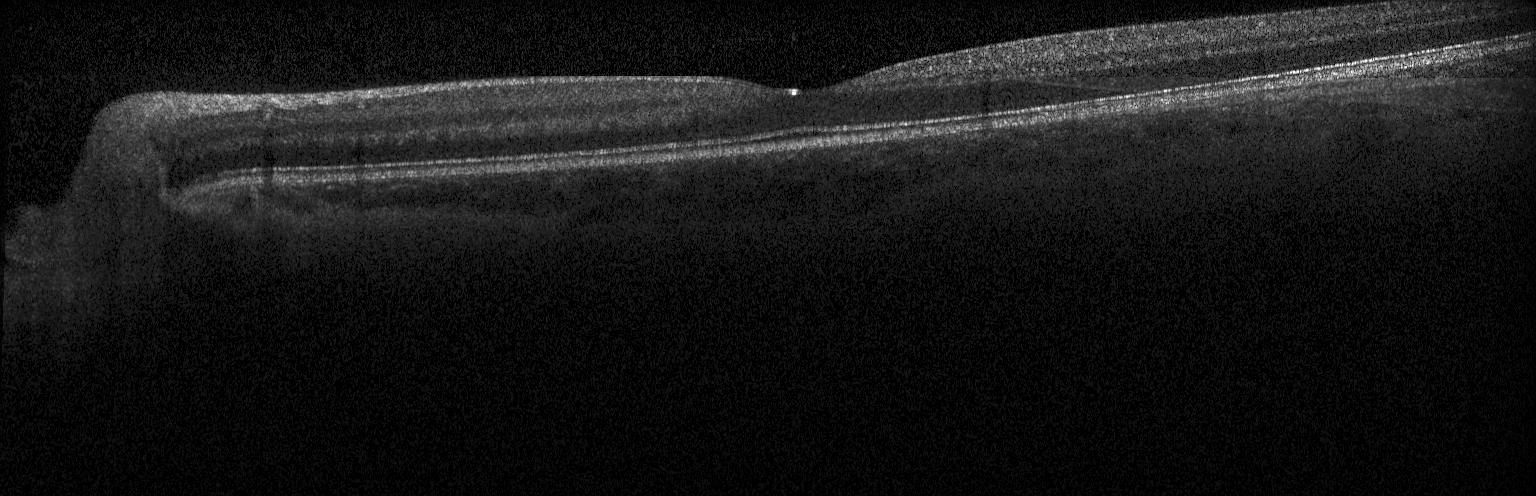
Heidelberg Spectralis OCT system. OCT B-scan
No choroidal neovascularization, diabetic macular edema, or drusen.